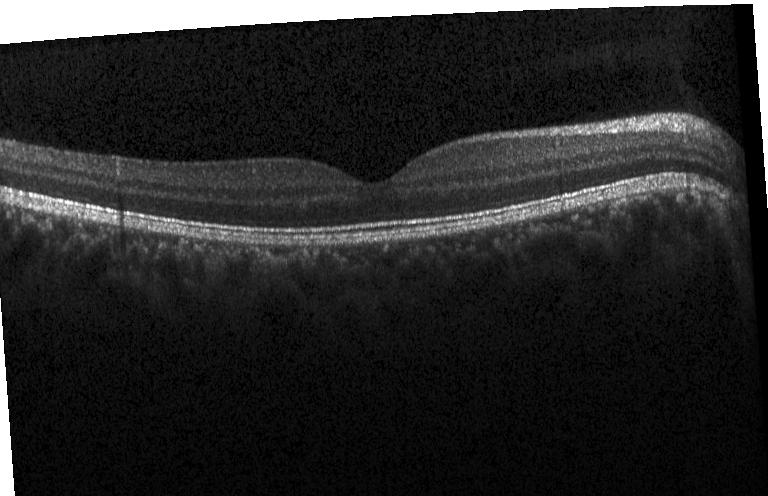
Spectral-domain OCT · OCT B-scan · instrument: Heidelberg Spectralis — This B-scan demonstrates no choroidal neovascularization, no diabetic macular edema, and no drusen.